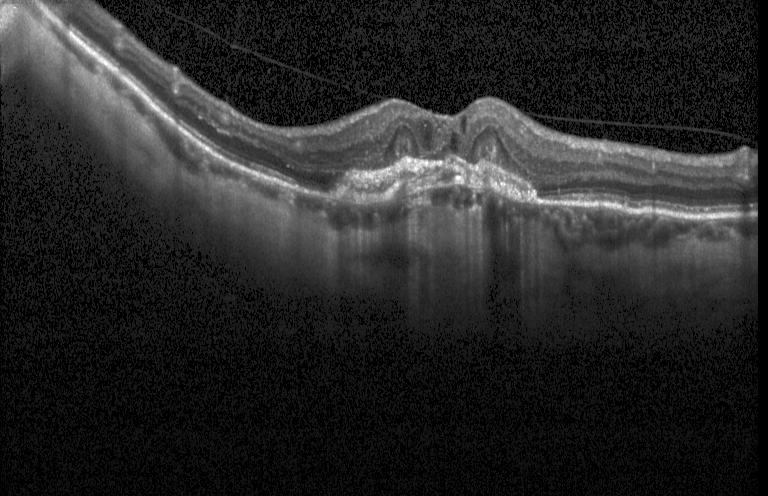
Optical coherence tomography B-scan, SD-OCT, instrument: Heidelberg Spectralis, fovea-centered. Diagnosis: CNV.